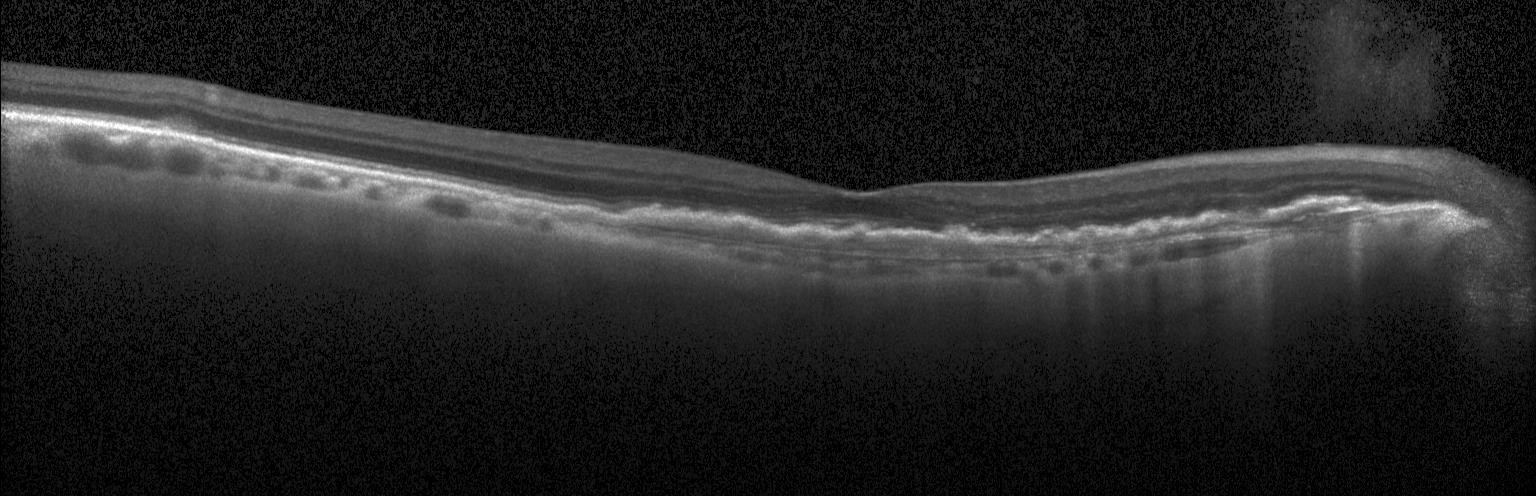 OCT scan showing a choroidal neovascular membrane.